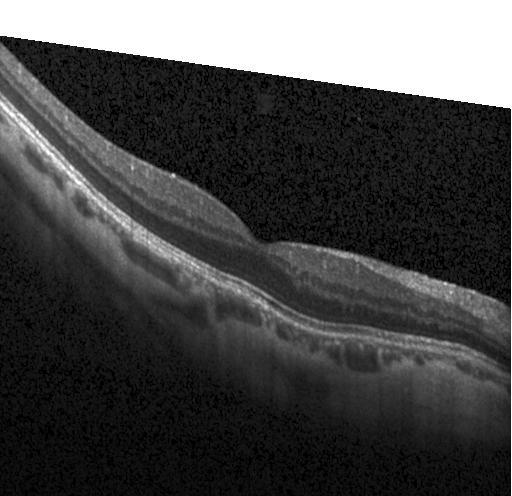
Macular OCT demonstrating no choroidal neovascularization, no diabetic macular edema, and no drusen.